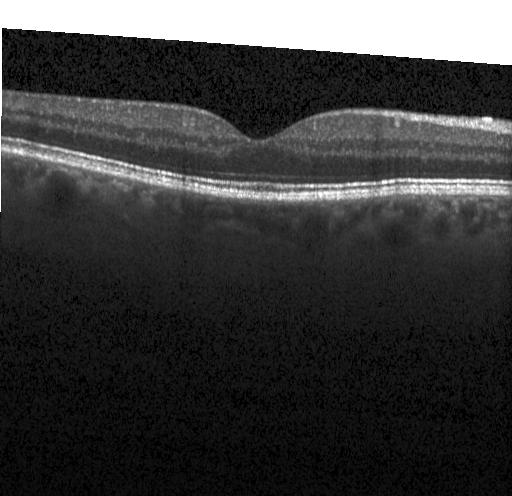
Macular scan, spectral-domain optical coherence tomography, optical coherence tomography B-scan
Dx: neither choroidal neovascularization, diabetic macular edema, nor drusen.